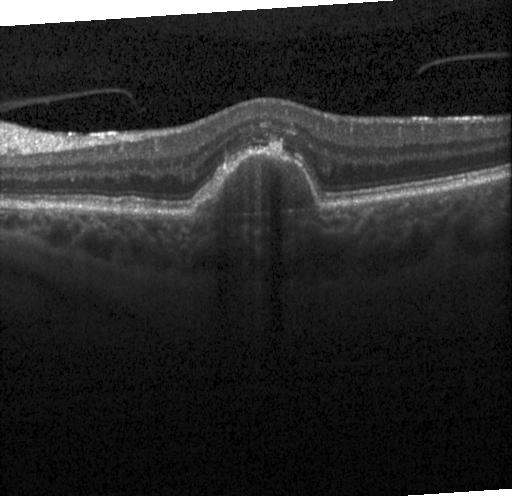 Optical coherence tomography B-scan. CNV.